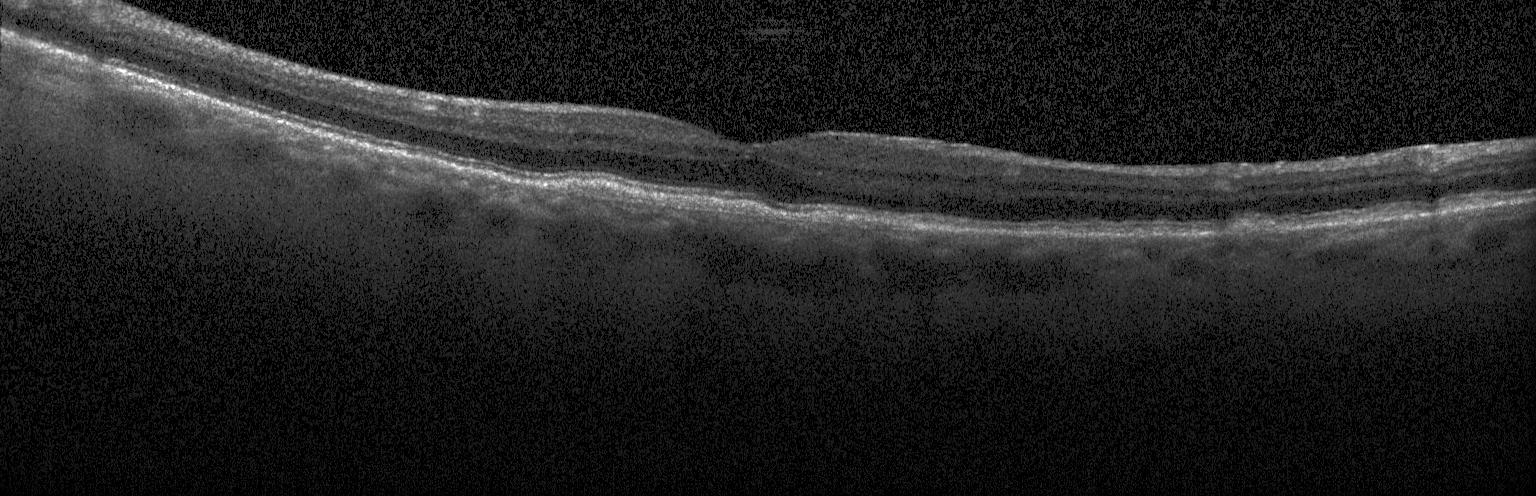

Centered on the fovea. SD-OCT. Retinal OCT B-scan. Heidelberg Spectralis OCT system — Finding: choroidal neovascularization.